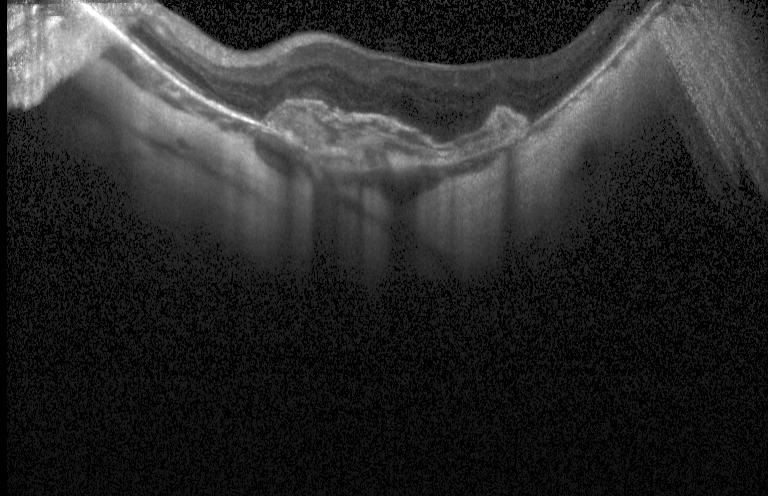
OCT line scan · horizontal scan through the fovea · Heidelberg Spectralis · SD-OCT. Impression: a choroidal neovascular membrane.